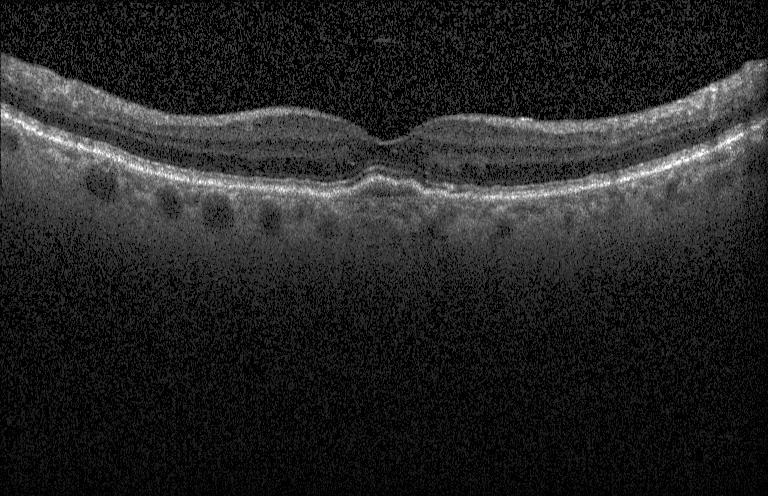
Fovea-centered, retinal OCT B-scan, instrument: Heidelberg Spectralis, spectral-domain optical coherence tomography.
Assessment: a choroidal neovascular membrane.